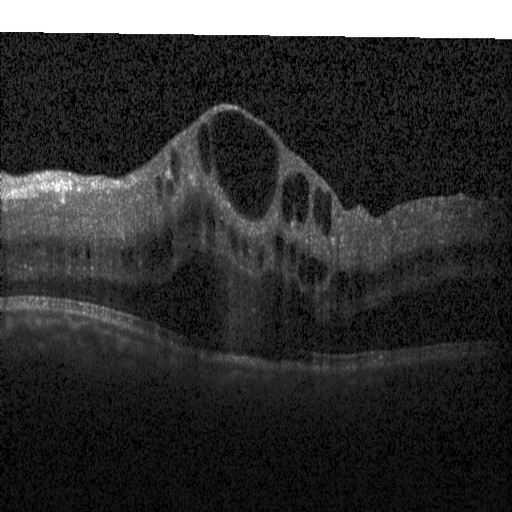
OCT line scan — Finding: diabetic macular edema (DME).